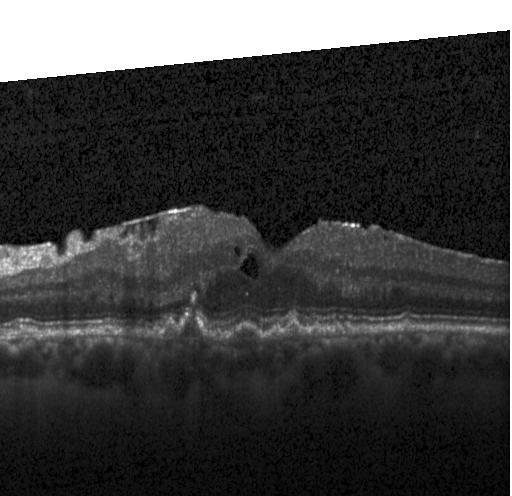
Finding: choroidal neovascularization (CNV).